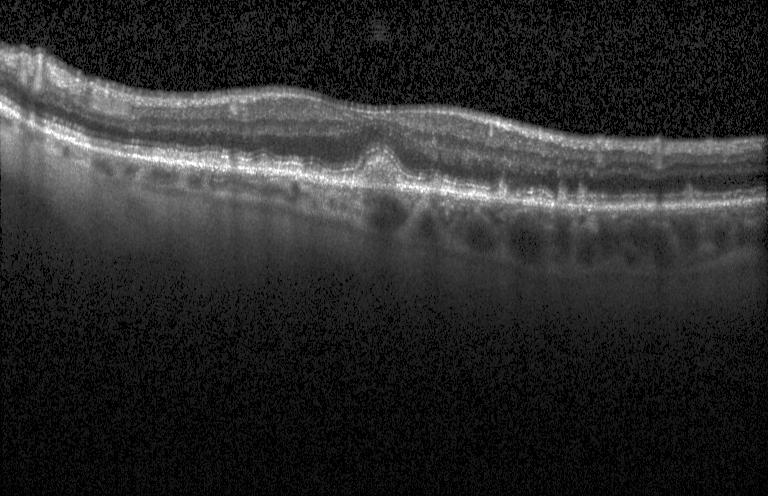

Optical coherence tomography B-scan. Finding: a choroidal neovascular membrane.